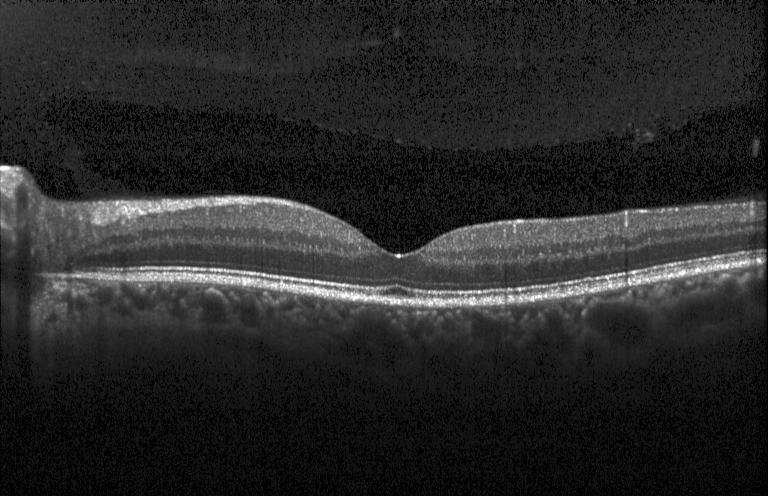 Heidelberg Spectralis OCT system. Through the macula. Optical coherence tomography scan — Finding: neither choroidal neovascularization, diabetic macular edema, nor drusen.